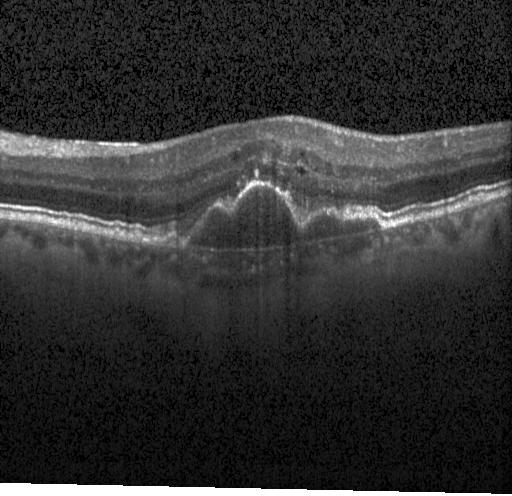

Optical coherence tomography scan
Diagnosis: a choroidal neovascular membrane.